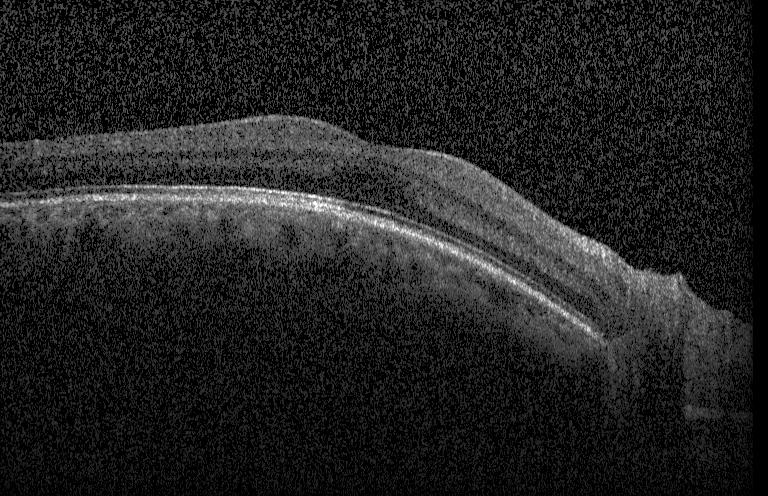

Heidelberg Spectralis · optical coherence tomography scan · centered on the fovea
Impression: no choroidal neovascularization, no diabetic macular edema, and no drusen.